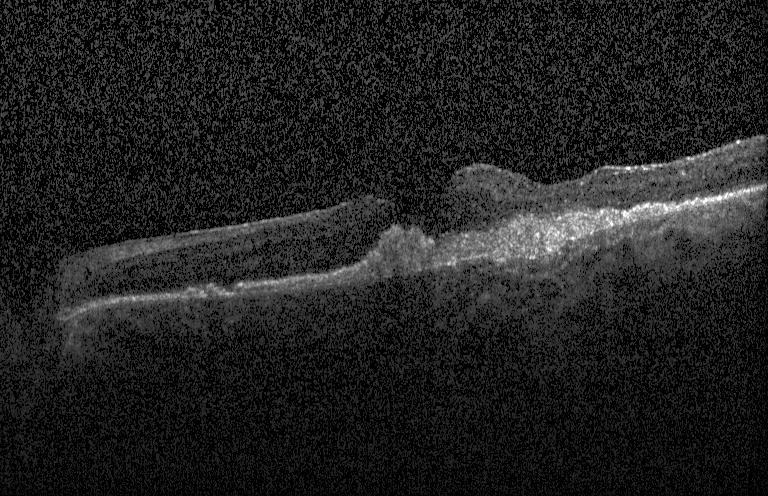

Macular OCT: choroidal neovascularization (CNV).